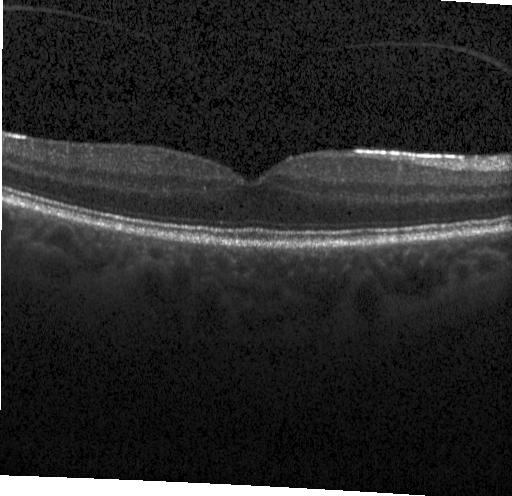

Macular OCT: no CNV, no DME, and no drusen.